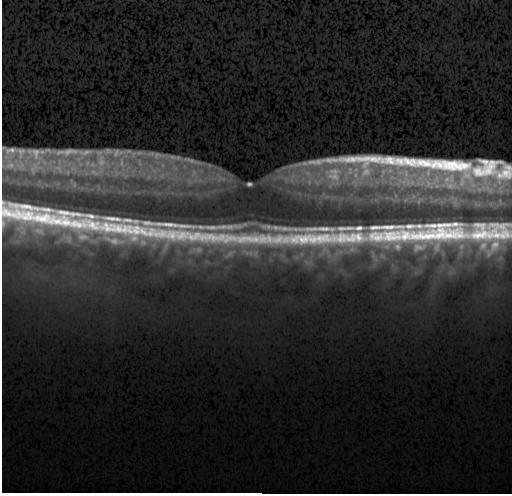 Retinal OCT B-scan · instrument: Heidelberg Spectralis · centered on the fovea · SD-OCT
Impression: no evidence of choroidal neovascularization, diabetic macular edema, or drusen.